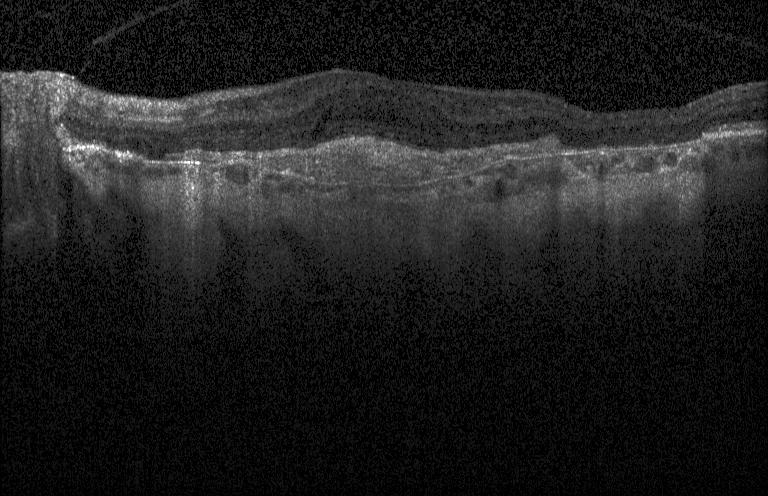 Instrument: Heidelberg Spectralis. Retinal OCT cross-section. Horizontal scan through the fovea
Impression: a choroidal neovascular membrane.